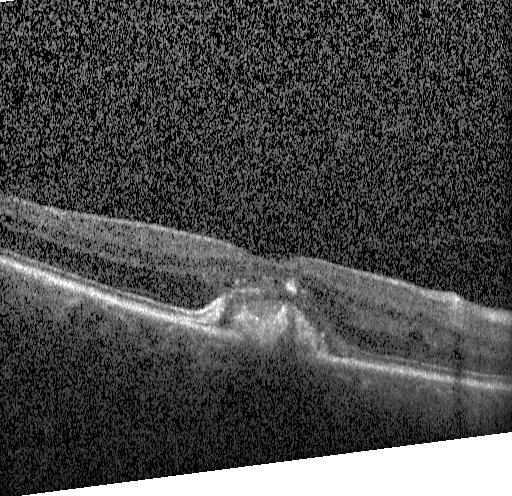
Retinal OCT B-scan
The scan shows a choroidal neovascular membrane.